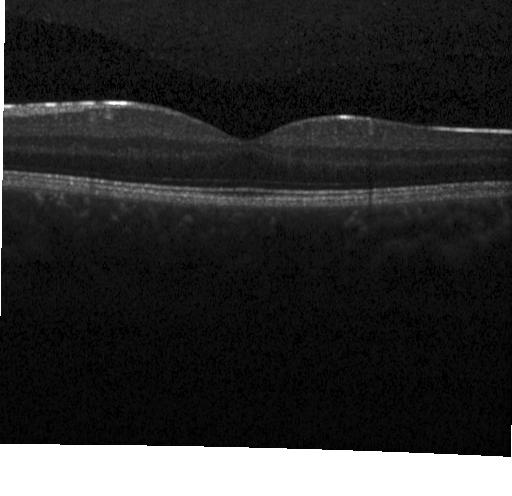 No evidence of choroidal neovascularization, diabetic macular edema, or drusen.